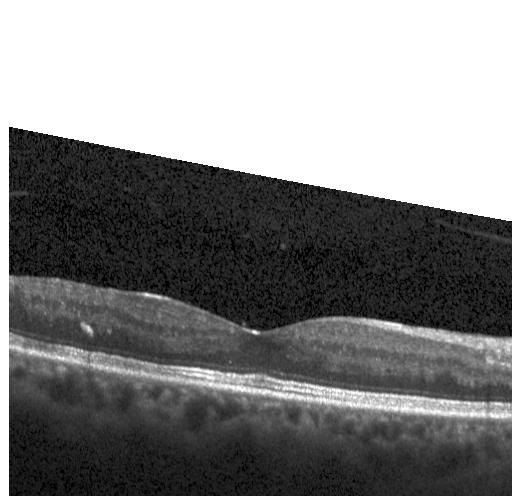 Heidelberg Spectralis OCT system. OCT B-scan. SD-OCT. Macular scan. Diagnosis: DME.